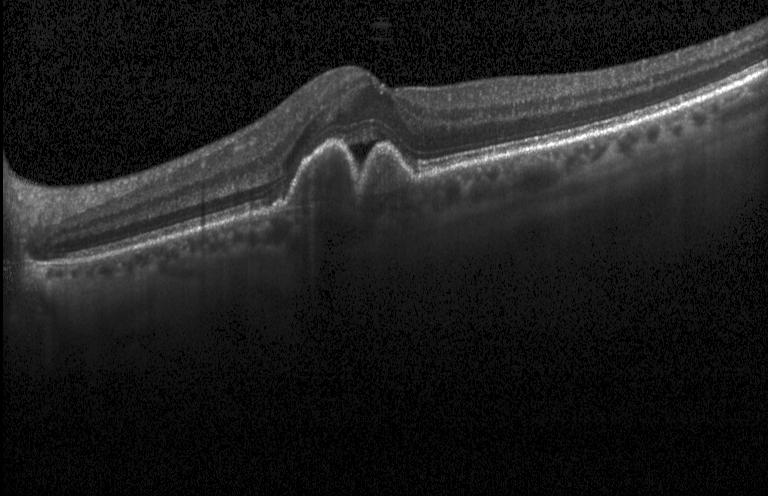
Optical coherence tomography B-scan. The scan shows choroidal neovascularization.